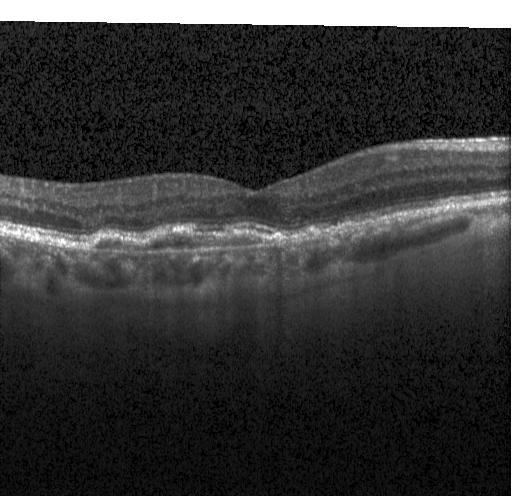 Retinal OCT cross-section. The scan shows a choroidal neovascular membrane.